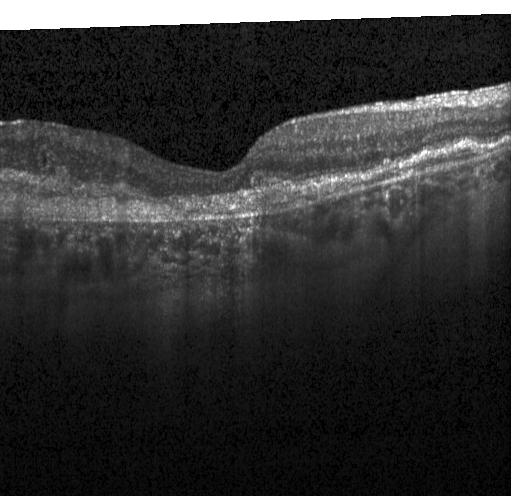

Heidelberg Spectralis OCT system · optical coherence tomography scan · spectral-domain OCT
Diagnosis: a choroidal neovascular membrane.